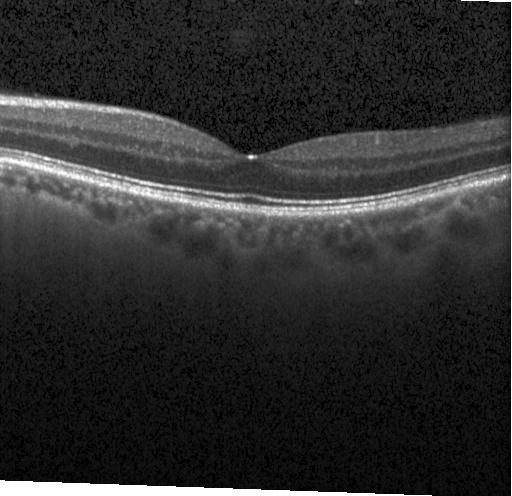
Optical coherence tomography B-scan. Impression: no evidence of CNV, DME, or drusen.